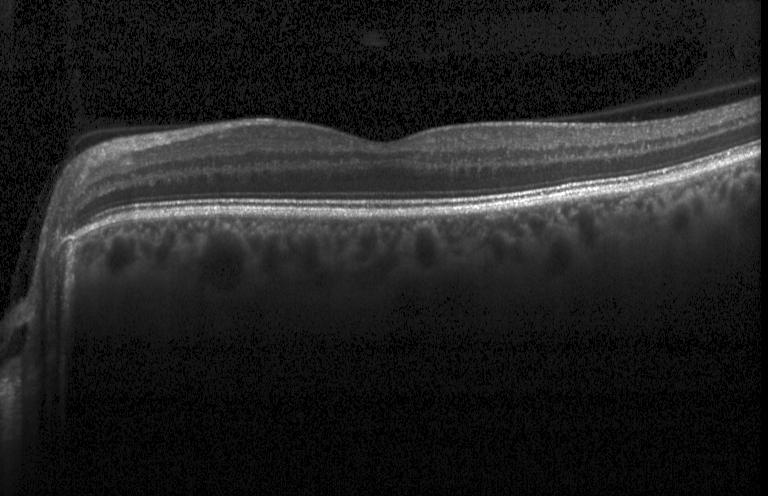

Horizontal scan through the fovea. Spectral-domain OCT. Heidelberg Spectralis. Retinal OCT B-scan.
Assessment: no CNV, DME, or drusen.